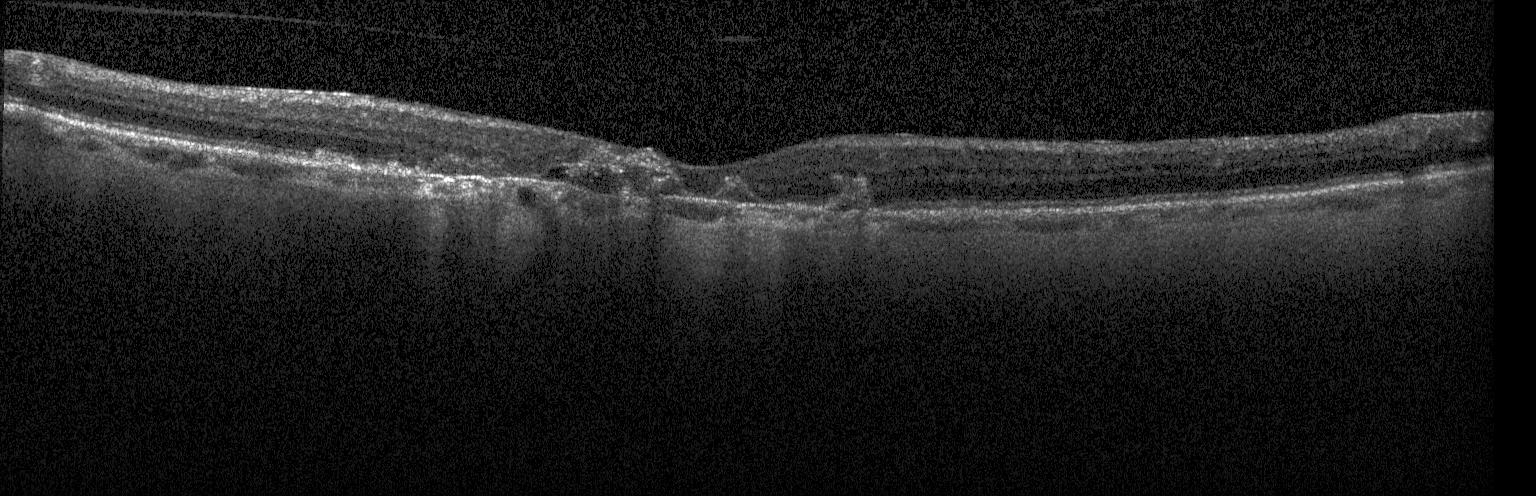
Fovea-centered · OCT B-scan — Dx: choroidal neovascularization (CNV).